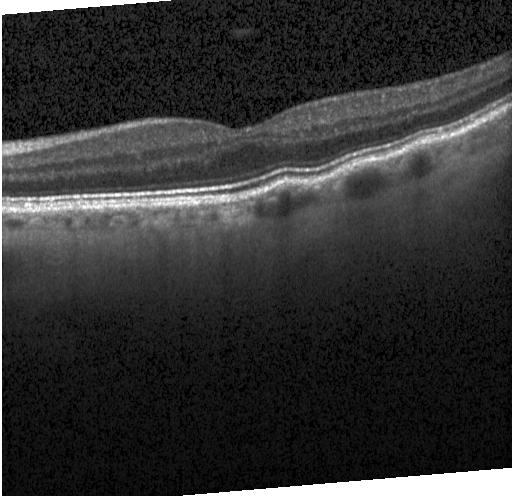 Heidelberg Spectralis · retinal OCT B-scan · SD-OCT · centered on the fovea — No choroidal neovascularization, no diabetic macular edema, and no drusen.